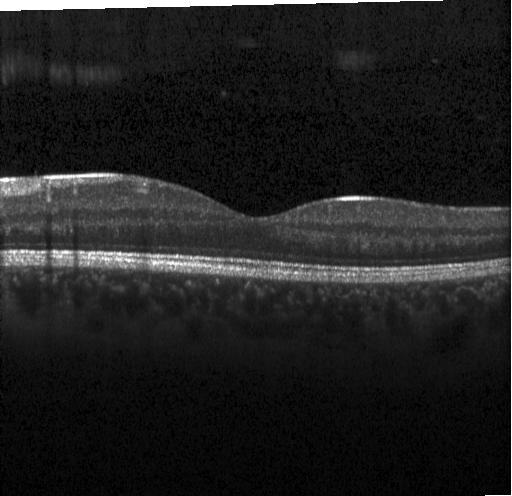
Fovea-centered · retinal OCT B-scan
Assessment: no CNV, no DME, and no drusen.